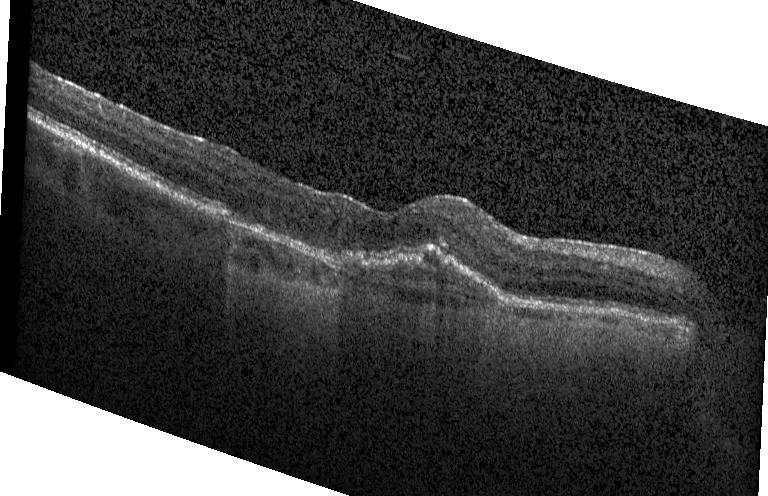

Diagnosis: CNV.